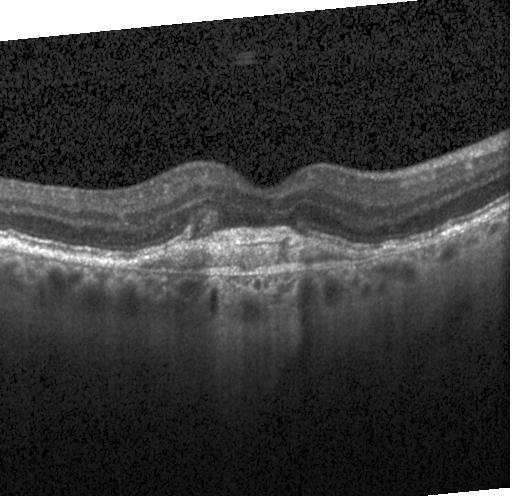 Impression: a choroidal neovascular membrane.